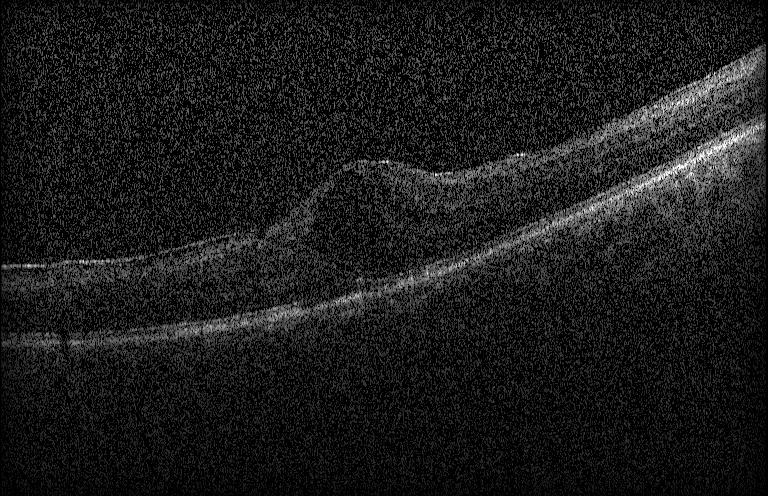 Dx: diabetic macular edema.